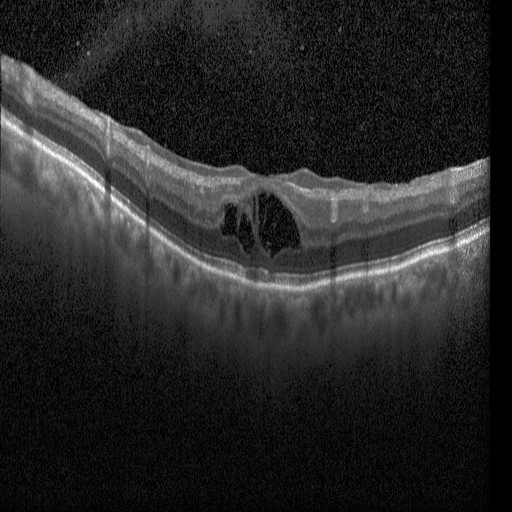 Finding: diabetic macular edema (DME).